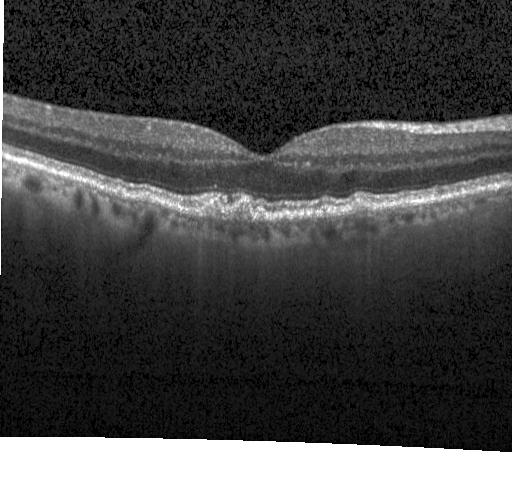 Optical coherence tomography scan, macular scan
Sub-RPE drusenoid deposits.